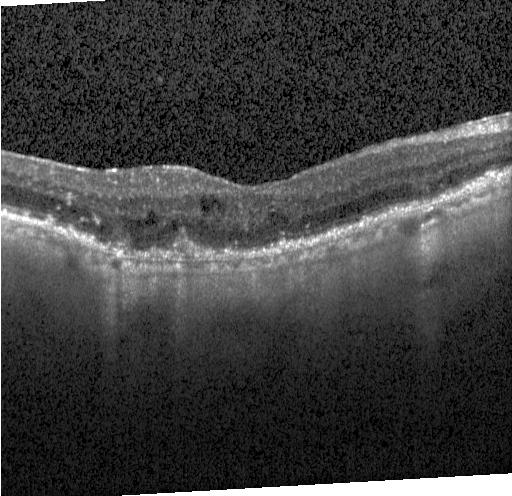 Retinal OCT B-scan. Spectral-domain optical coherence tomography. Finding: a choroidal neovascular membrane.